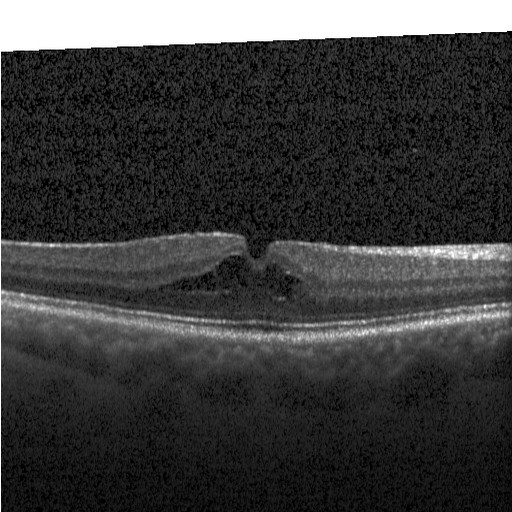
OCT B-scan — Impression: diabetic macular edema (DME).